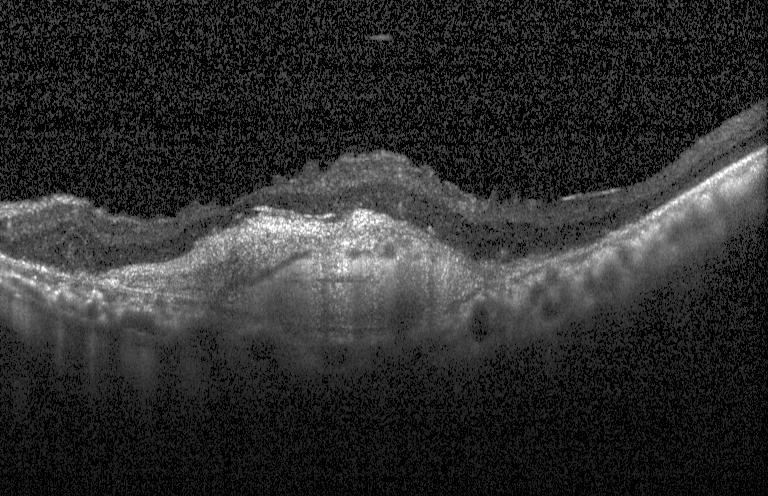
OCT scan showing CNV.